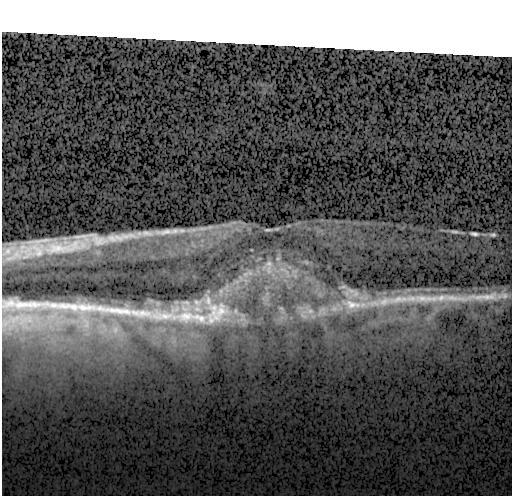
Heidelberg Spectralis OCT system; spectral-domain optical coherence tomography; optical coherence tomography B-scan
Impression: a choroidal neovascular membrane.